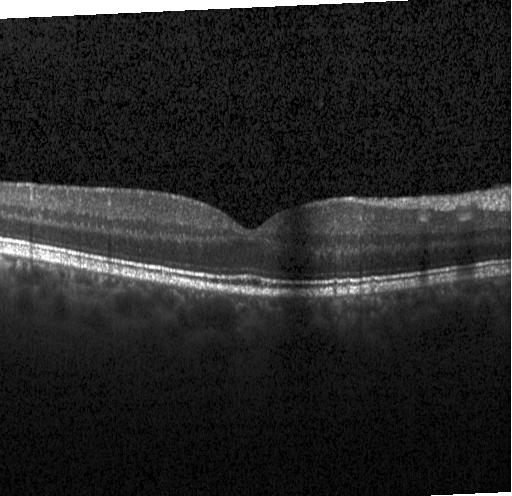
Heidelberg Spectralis OCT system. Retinal OCT B-scan. Spectral-domain OCT.
Finding: no choroidal neovascularization, diabetic macular edema, or drusen.